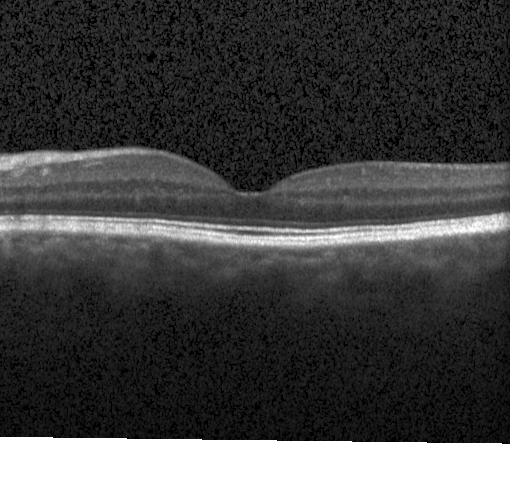 Finding: neither choroidal neovascularization, diabetic macular edema, nor drusen.